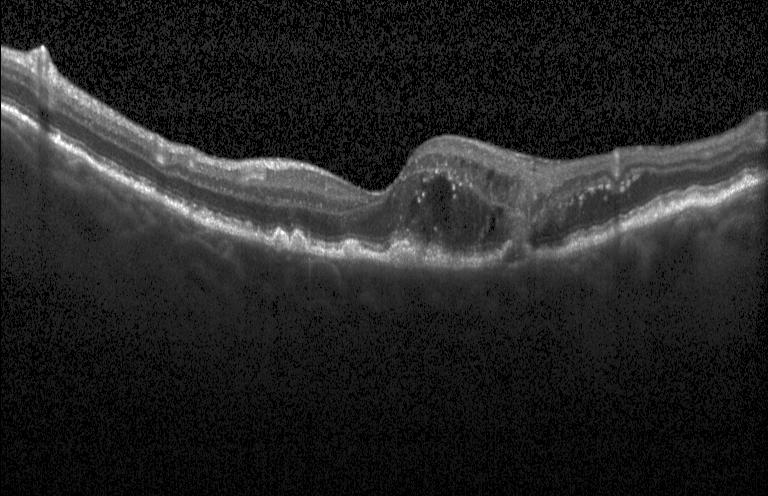

This B-scan demonstrates choroidal neovascularization (CNV).